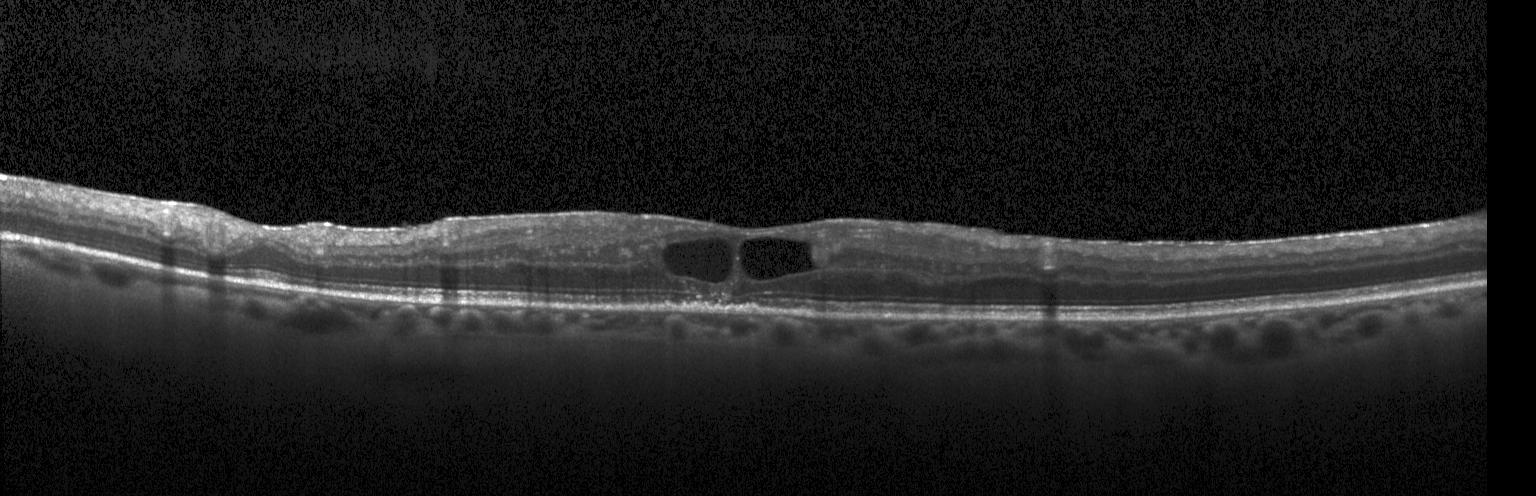 OCT finding: diabetic macular edema.